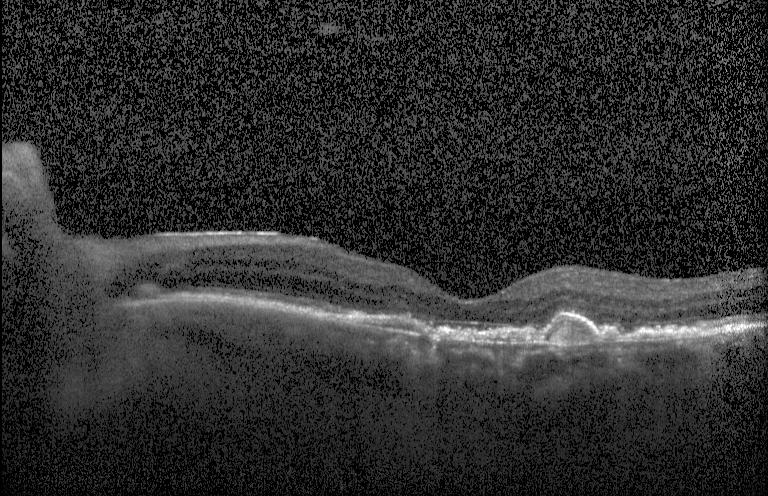 Optical coherence tomography scan
Finding: a choroidal neovascular membrane.